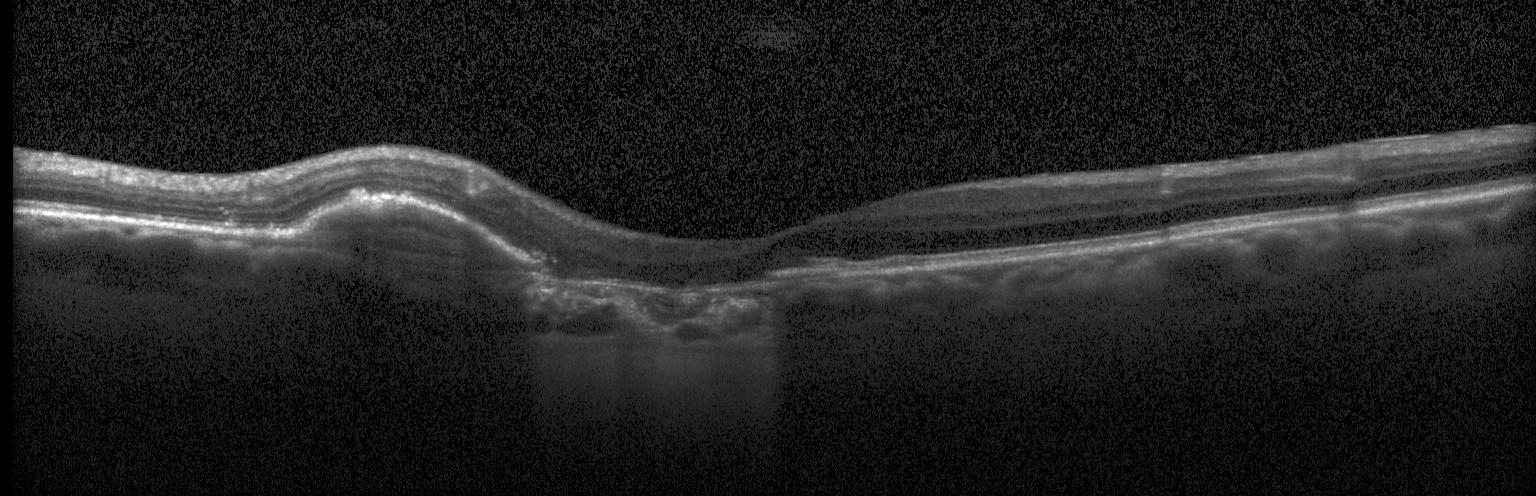

Instrument: Heidelberg Spectralis · OCT B-scan · through the macula · spectral-domain optical coherence tomography.
CNV.